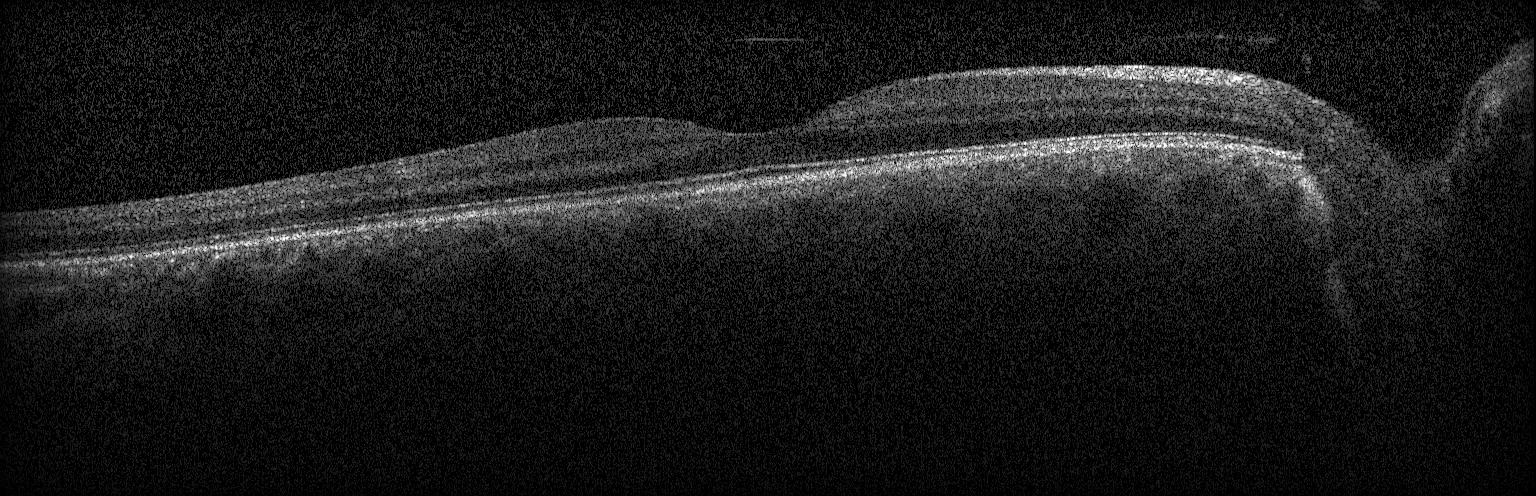

Optical coherence tomography B-scan.
Dx: no evidence of choroidal neovascularization, diabetic macular edema, or drusen.